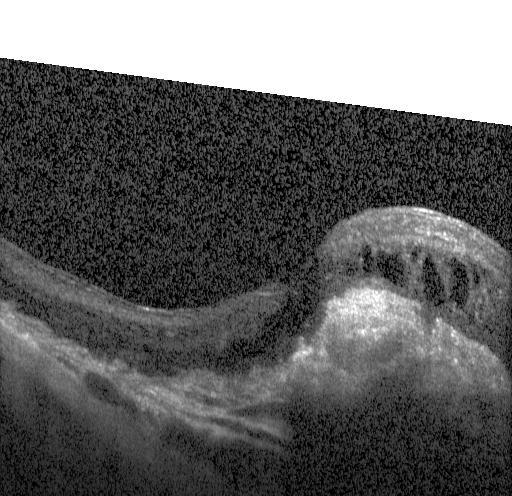

OCT B-scan showing choroidal neovascularization.